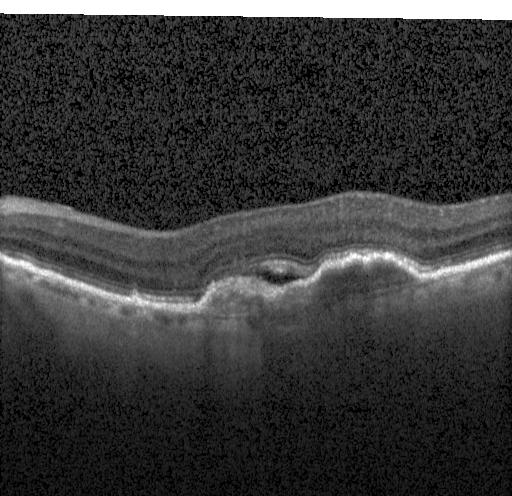

Retinal OCT B-scan. Dx: a choroidal neovascular membrane.